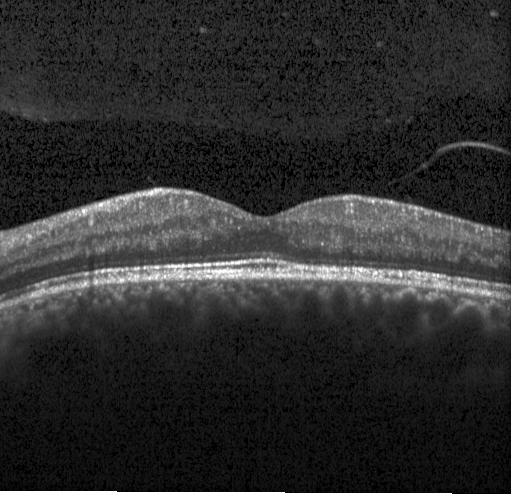 Centered on the fovea, OCT B-scan.
The scan shows no evidence of CNV, DME, or drusen.